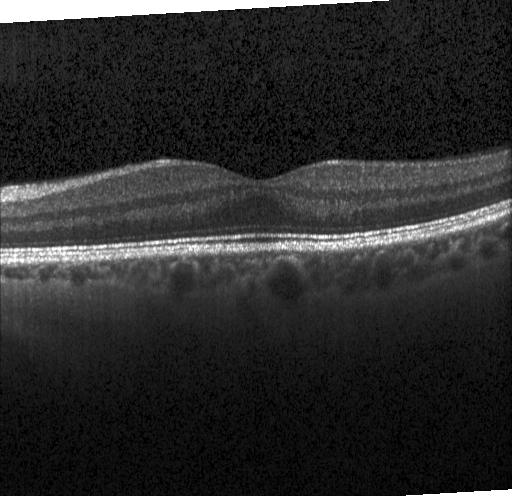

Through the macula · SD-OCT · acquired on a Heidelberg Spectralis · optical coherence tomography B-scan.
Assessment: no evidence of CNV, DME, or drusen.